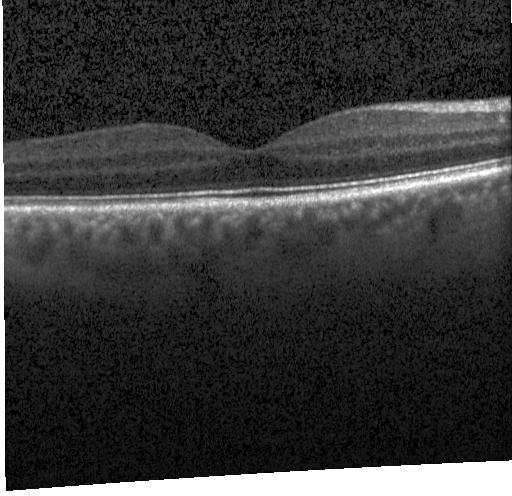
Retinal OCT B-scan; instrument: Heidelberg Spectralis; centered on the fovea; spectral-domain optical coherence tomography
The scan shows no CNV, DME, or drusen.